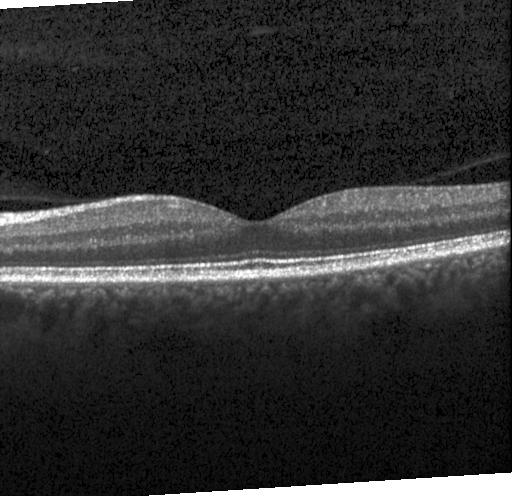

Acquired on a Heidelberg Spectralis. OCT B-scan. Spectral-domain optical coherence tomography. Centered on the fovea
Impression: no evidence of choroidal neovascularization, diabetic macular edema, or drusen.